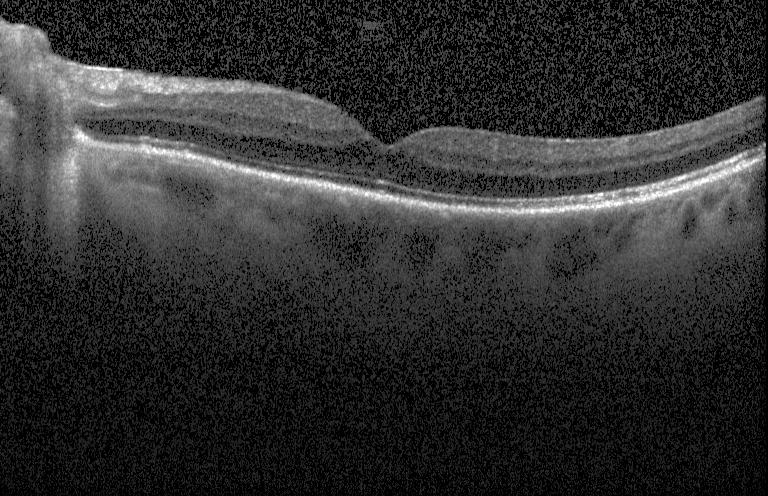

OCT B-scan — The scan shows no CNV, DME, or drusen.